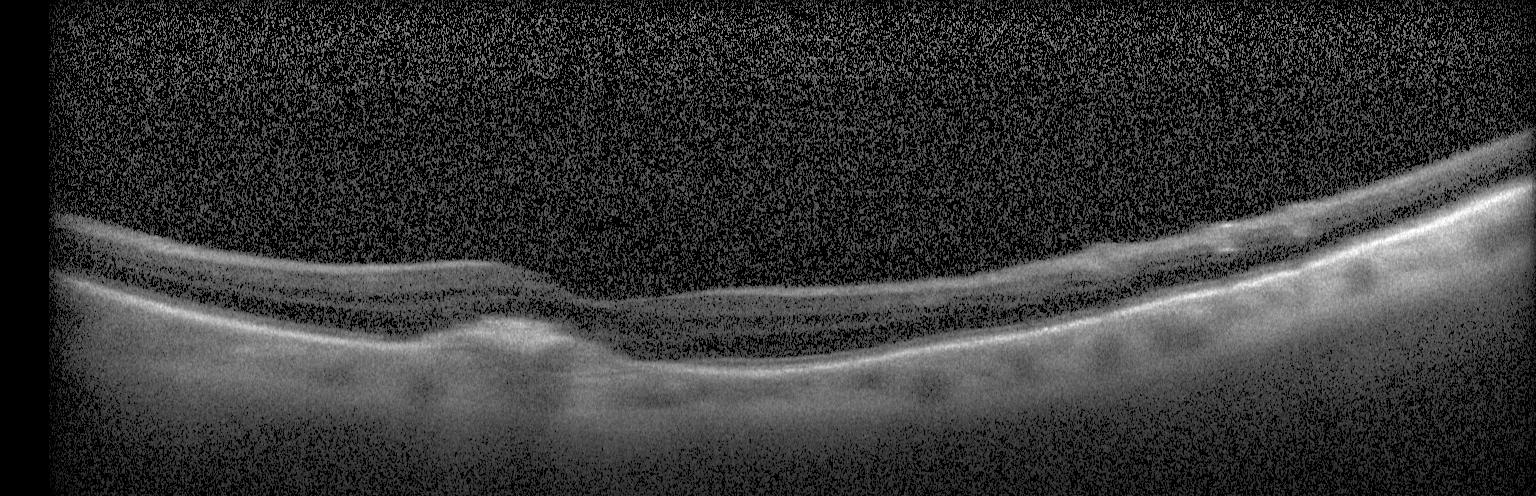 Macular OCT demonstrating a choroidal neovascular membrane.